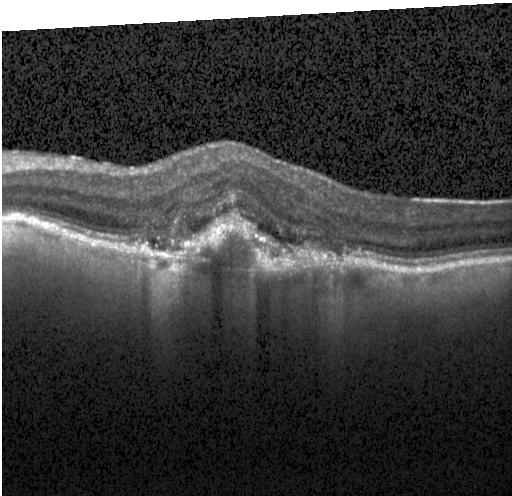
Horizontal scan through the fovea · retinal OCT B-scan
Diagnosis: a choroidal neovascular membrane.